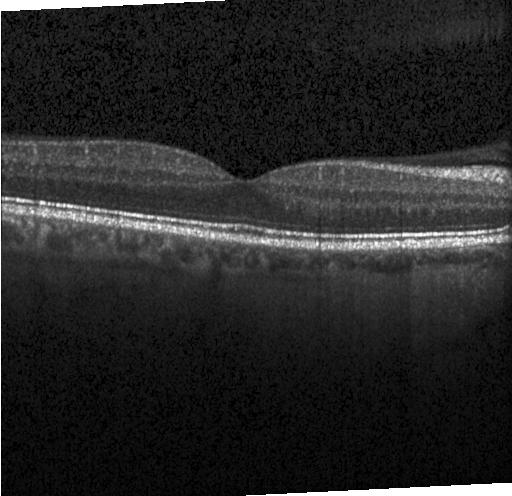
Assessment: no evidence of choroidal neovascularization, diabetic macular edema, or drusen.